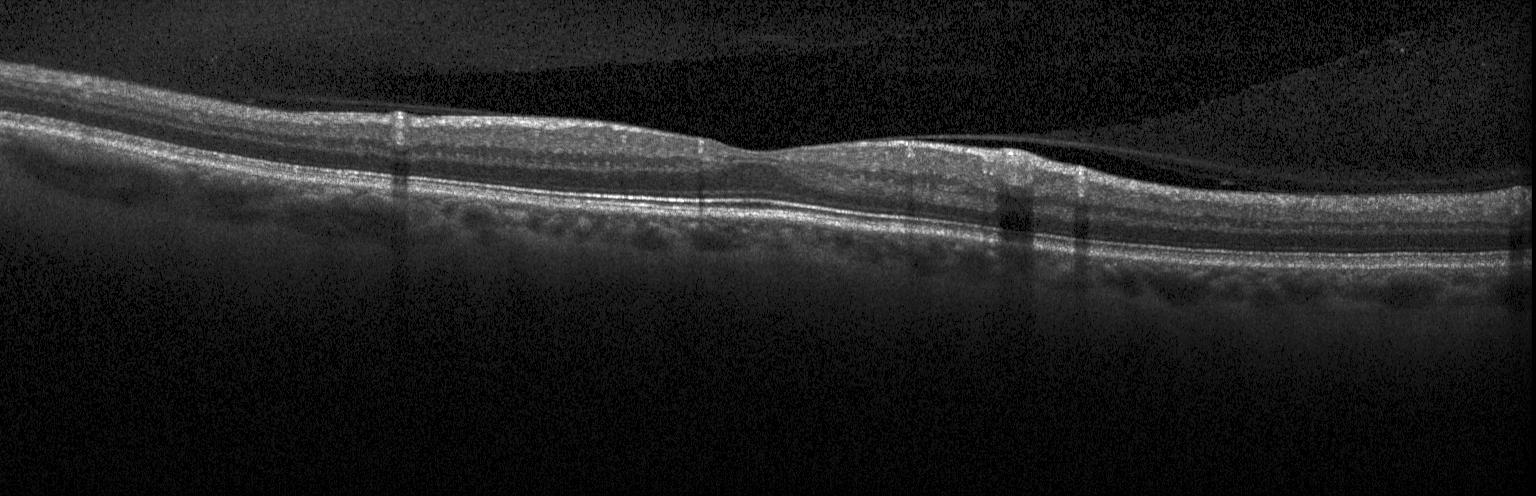 Optical coherence tomography scan. This B-scan demonstrates no evidence of choroidal neovascularization, diabetic macular edema, or drusen.